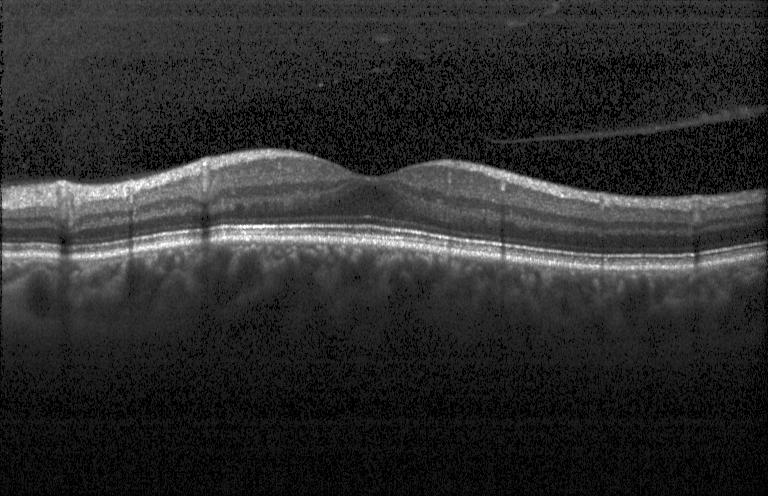

Macular OCT: no choroidal neovascularization, diabetic macular edema, or drusen.